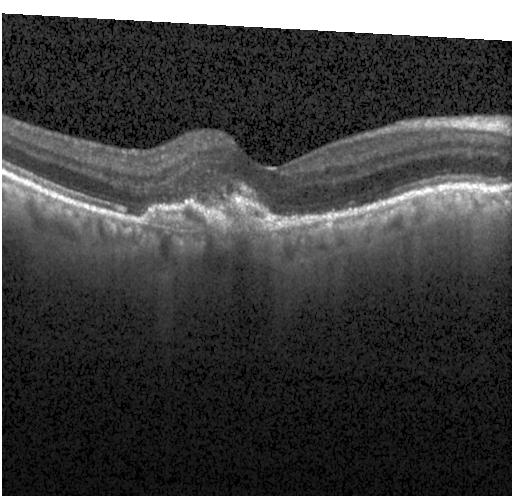

OCT finding: a choroidal neovascular membrane.